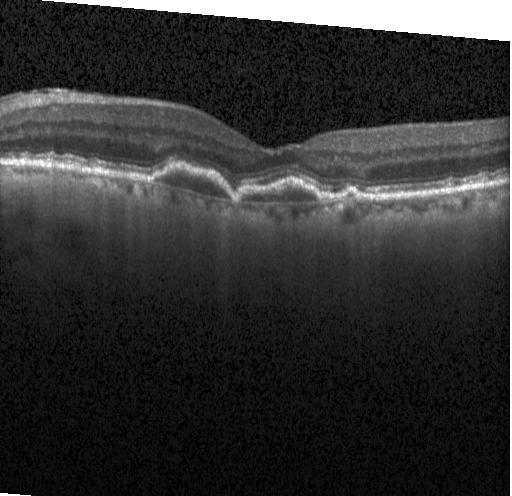
Retinal OCT cross-section — Macular OCT: CNV.